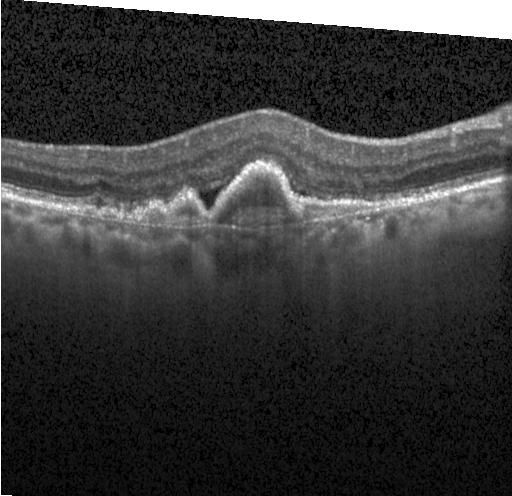
Spectral-domain OCT B-scan: a choroidal neovascular membrane.